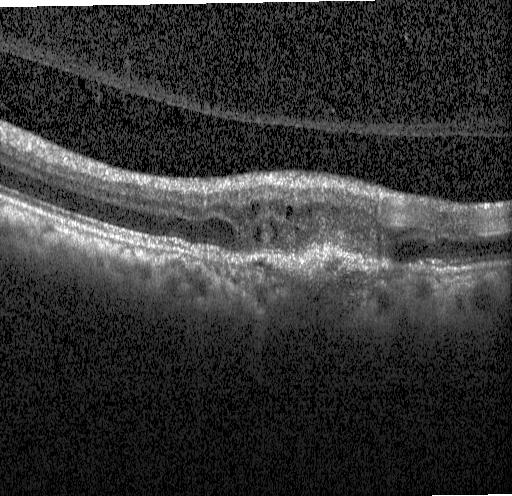
Optical coherence tomography B-scan. Impression: a choroidal neovascular membrane.